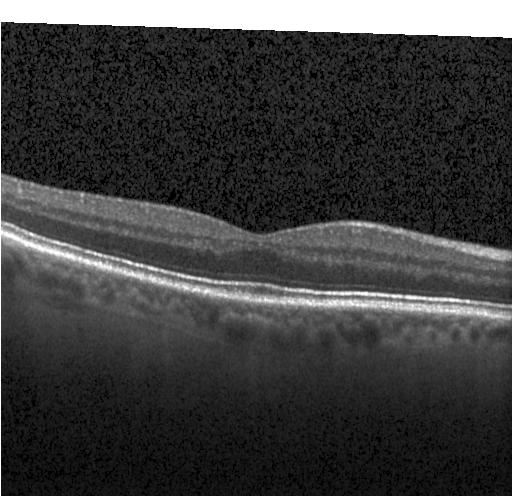 OCT B-scan; spectral-domain optical coherence tomography; through the macula. Assessment: no CNV, DME, or drusen.